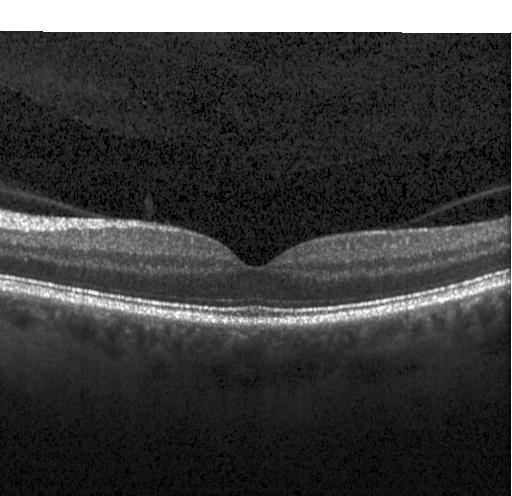
Retinal OCT cross-section showing no CNV, DME, or drusen.